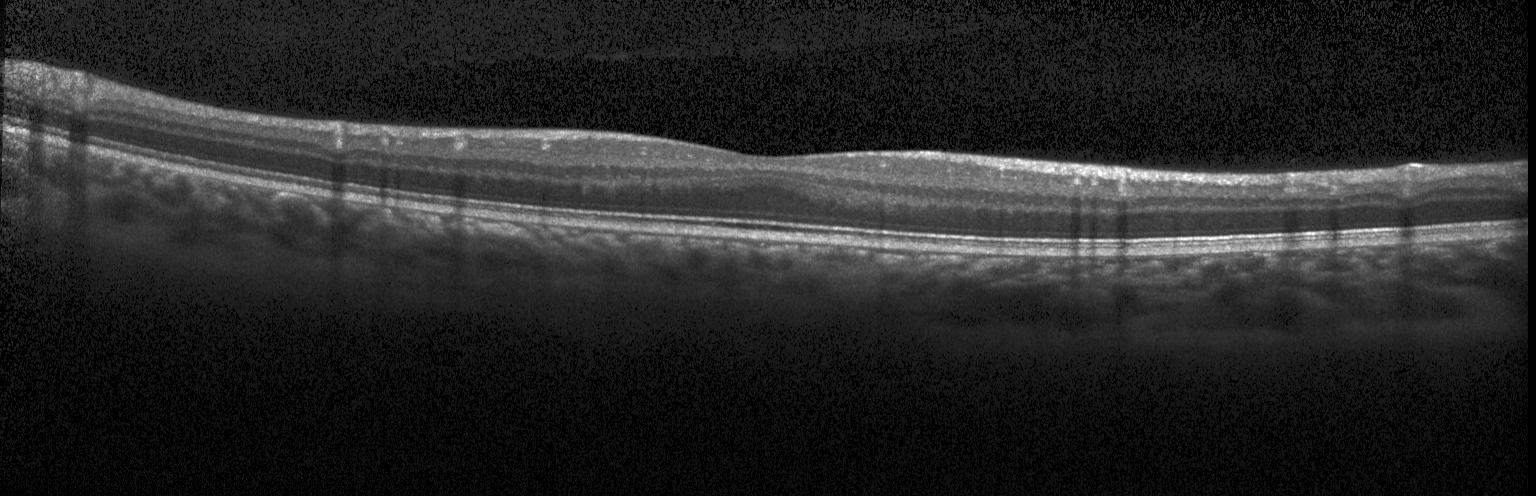

Retinal OCT cross-section — No choroidal neovascularization, diabetic macular edema, or drusen.